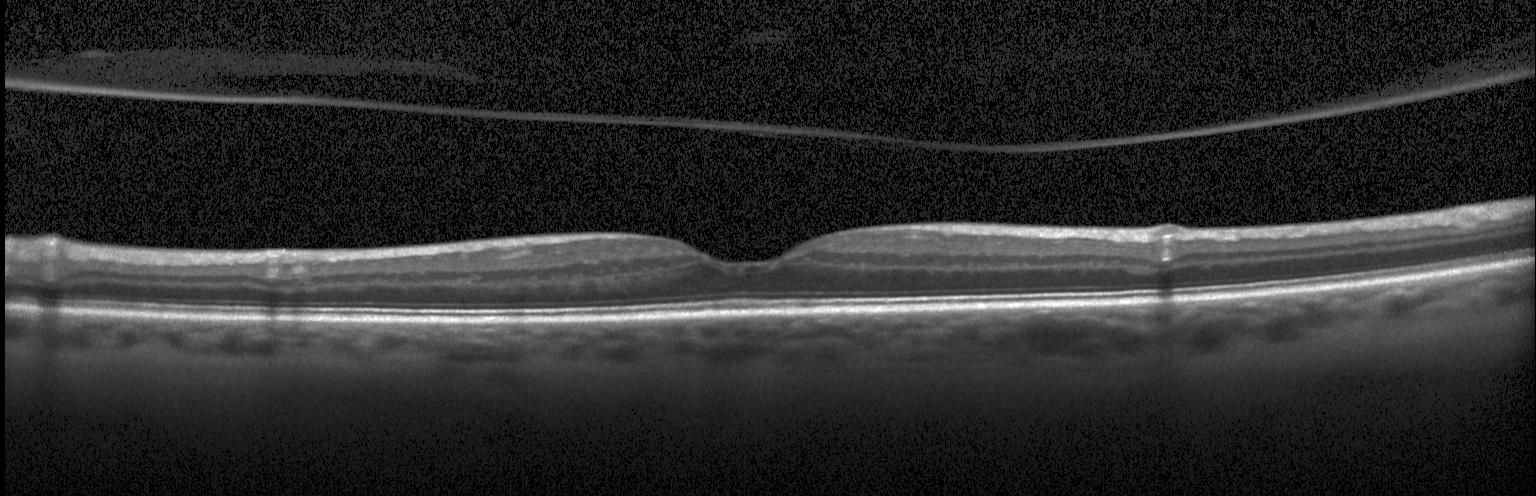

OCT finding: no choroidal neovascularization, no diabetic macular edema, and no drusen.